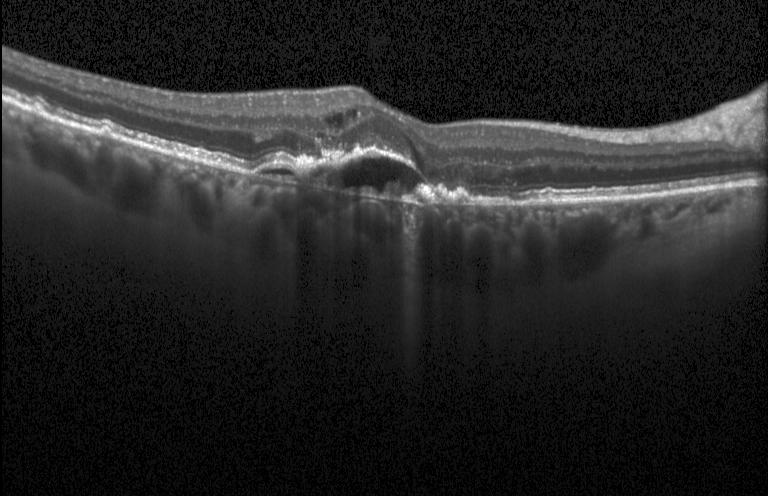

Choroidal neovascularization.